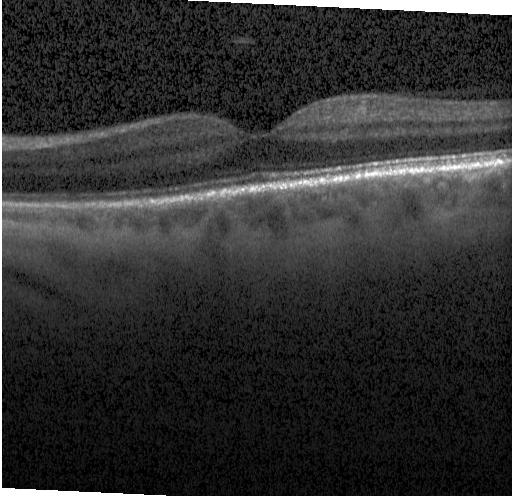 Retinal OCT cross-section. Impression: no evidence of choroidal neovascularization, diabetic macular edema, or drusen.